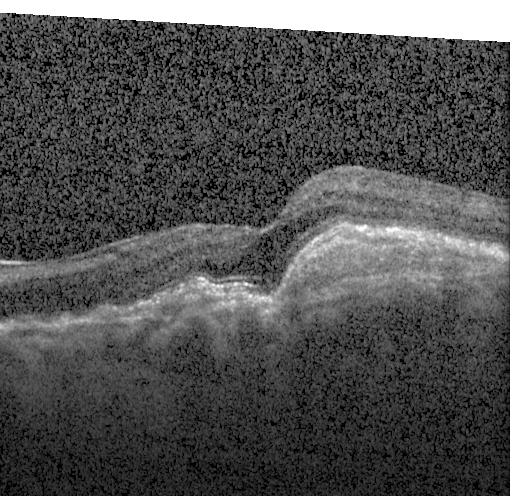 Finding: a choroidal neovascular membrane.